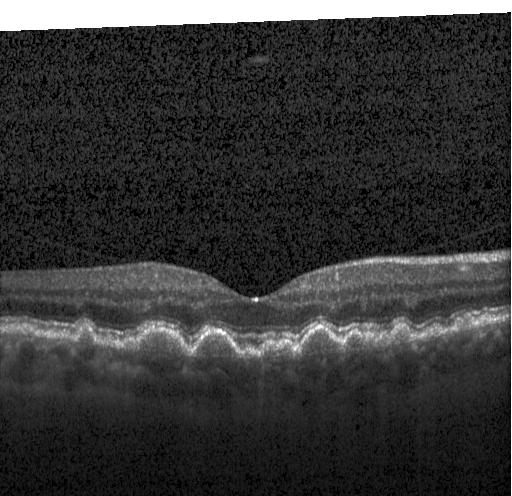 SD-OCT · OCT line scan — Diagnosis: sub-RPE drusenoid deposits.